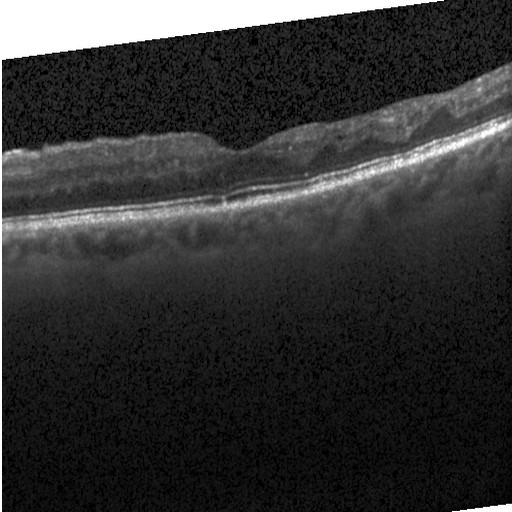 Optical coherence tomography B-scan
Finding: diabetic macular edema (DME).